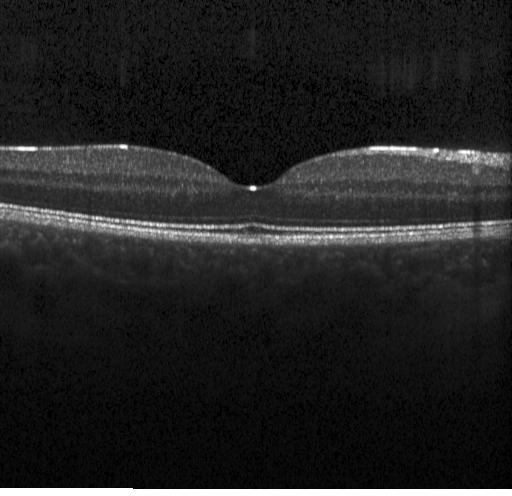
Heidelberg Spectralis. Horizontal scan through the fovea. Optical coherence tomography B-scan. Spectral-domain OCT
This B-scan demonstrates no CNV, no DME, and no drusen.